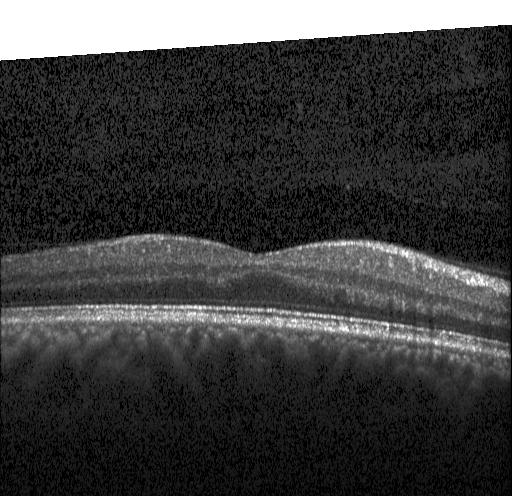

Retinal OCT cross-section
This B-scan demonstrates no CNV, no DME, and no drusen.